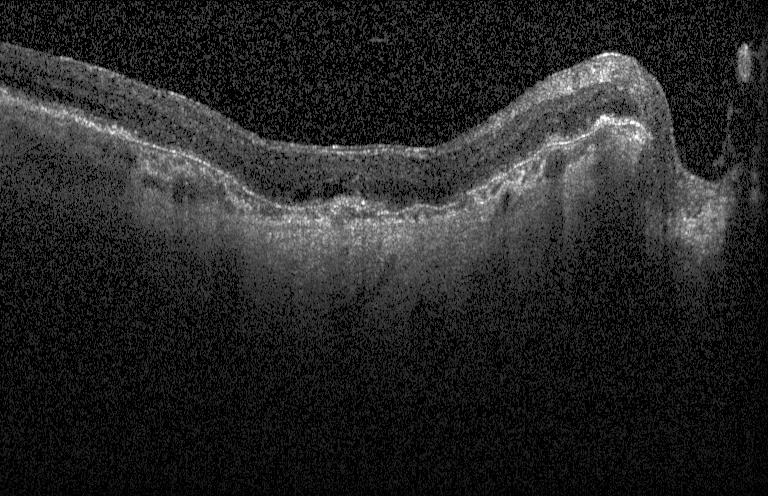 Optical coherence tomography scan · horizontal scan through the fovea · acquired on a Heidelberg Spectralis · spectral-domain OCT.
Finding: a choroidal neovascular membrane.